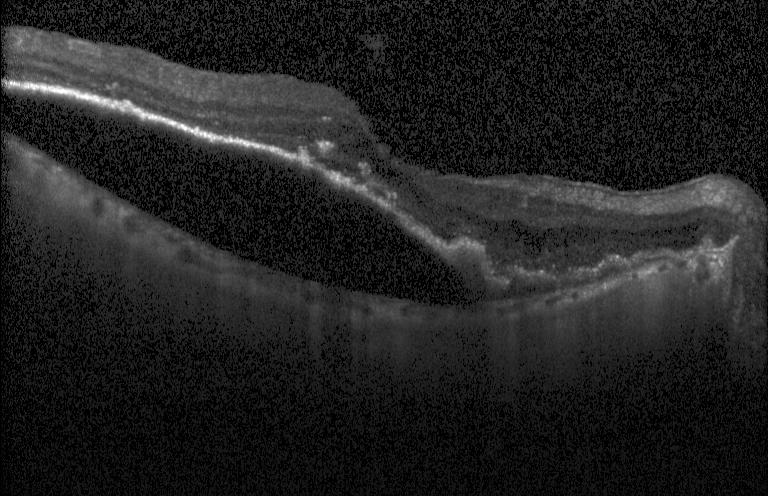
Assessment: CNV.